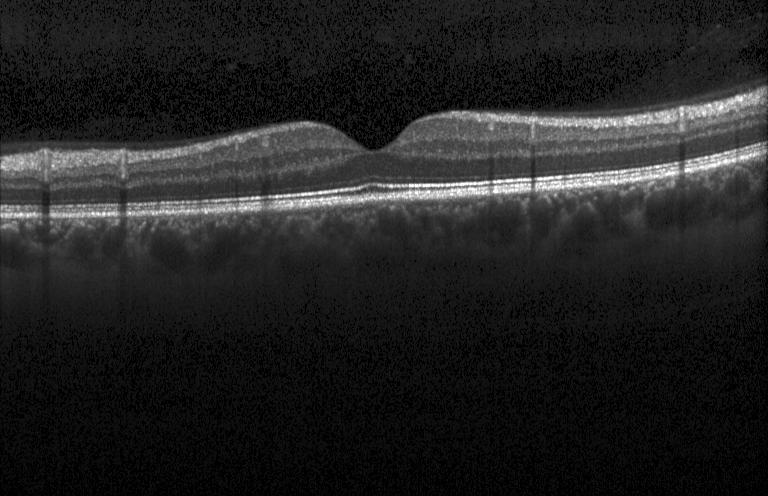
Optical coherence tomography scan; centered on the fovea
Finding: neither choroidal neovascularization, diabetic macular edema, nor drusen.